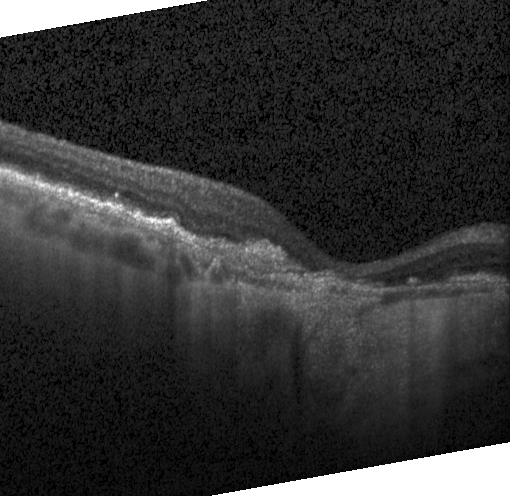 SD-OCT, retinal OCT B-scan.
Dx: CNV.